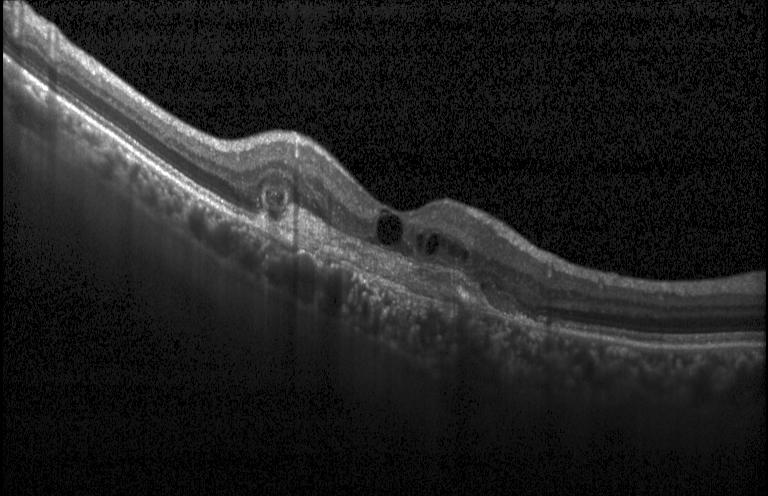
Spectral-domain optical coherence tomography. Retinal OCT B-scan — Impression: choroidal neovascularization (CNV).